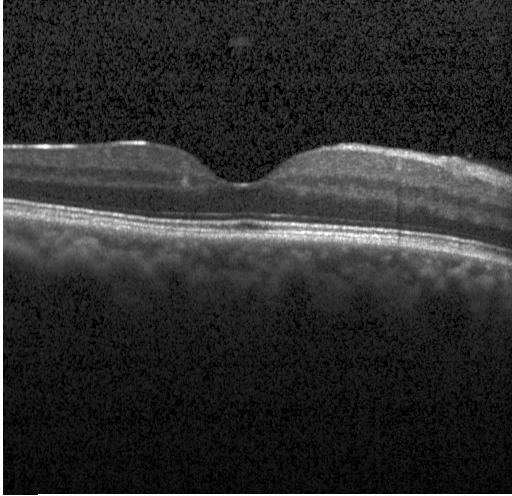

OCT B-scan. No choroidal neovascularization, no diabetic macular edema, and no drusen.